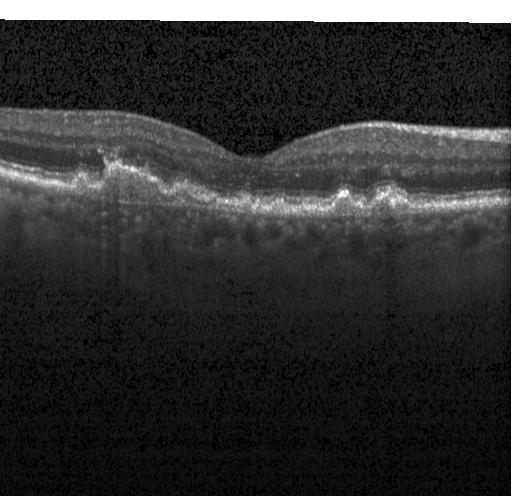

Acquired on a Heidelberg Spectralis, OCT line scan, centered on the fovea. Impression: choroidal neovascularization.